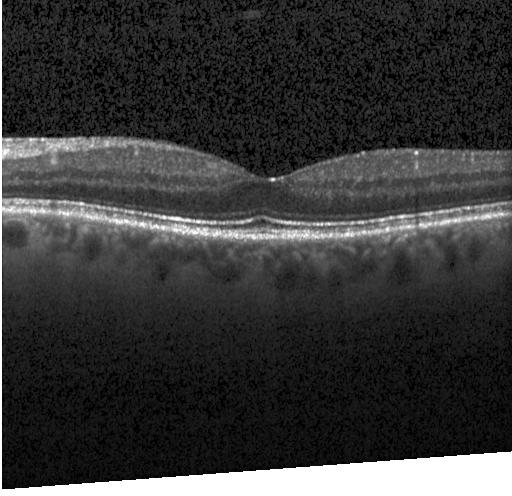

Instrument: Heidelberg Spectralis, retinal OCT B-scan. The scan shows neither choroidal neovascularization, diabetic macular edema, nor drusen.